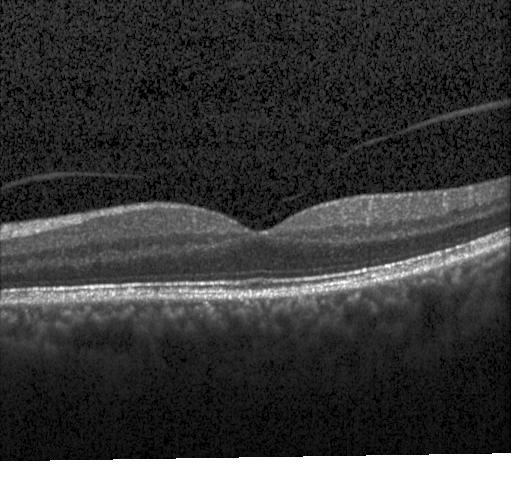 Acquired on a Heidelberg Spectralis. OCT B-scan
No evidence of CNV, DME, or drusen.